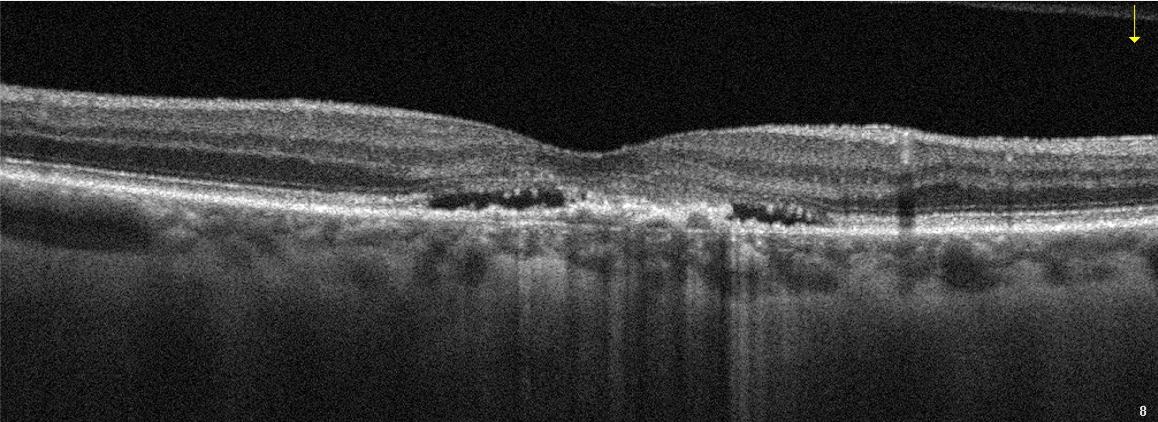 Optovue Avanti RTVue XR; retinal OCT B-scan; fovea-centered. Finding: age-related macular degeneration (AMD).